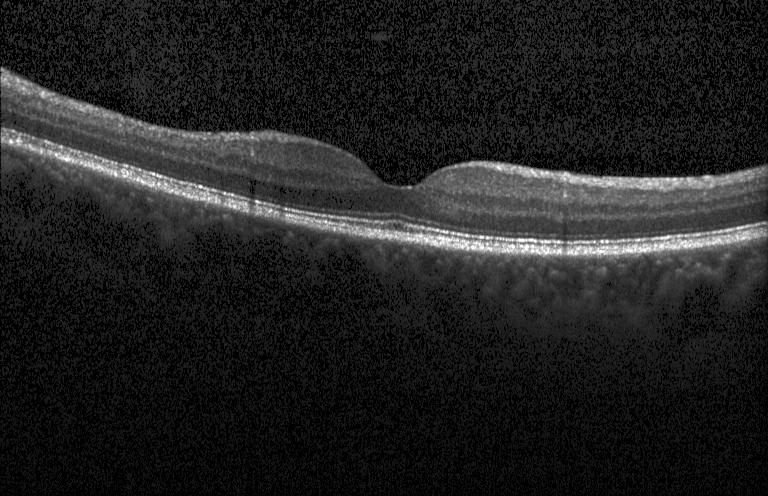
Retinal OCT cross-section — No choroidal neovascularization, diabetic macular edema, or drusen.